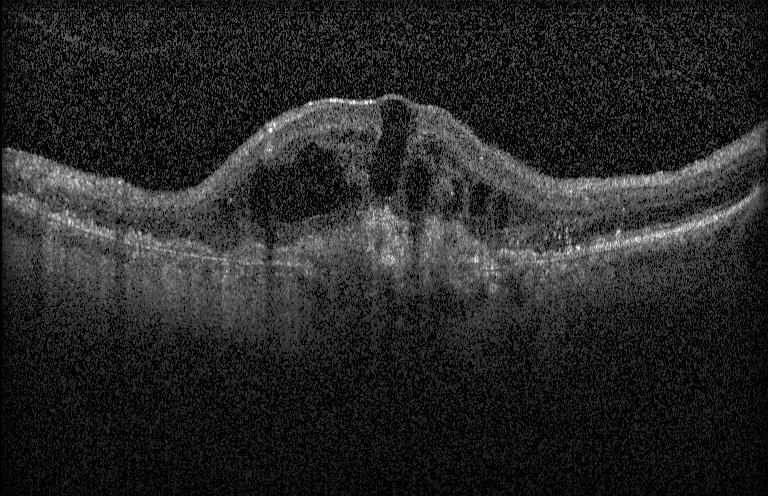 Heidelberg Spectralis · spectral-domain OCT · optical coherence tomography scan — CNV.